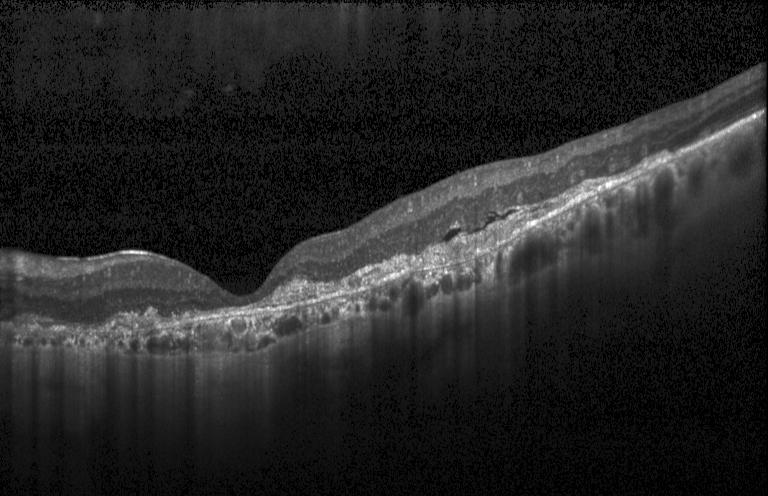 Heidelberg Spectralis · retinal OCT cross-section · spectral-domain OCT
Dx: a choroidal neovascular membrane.